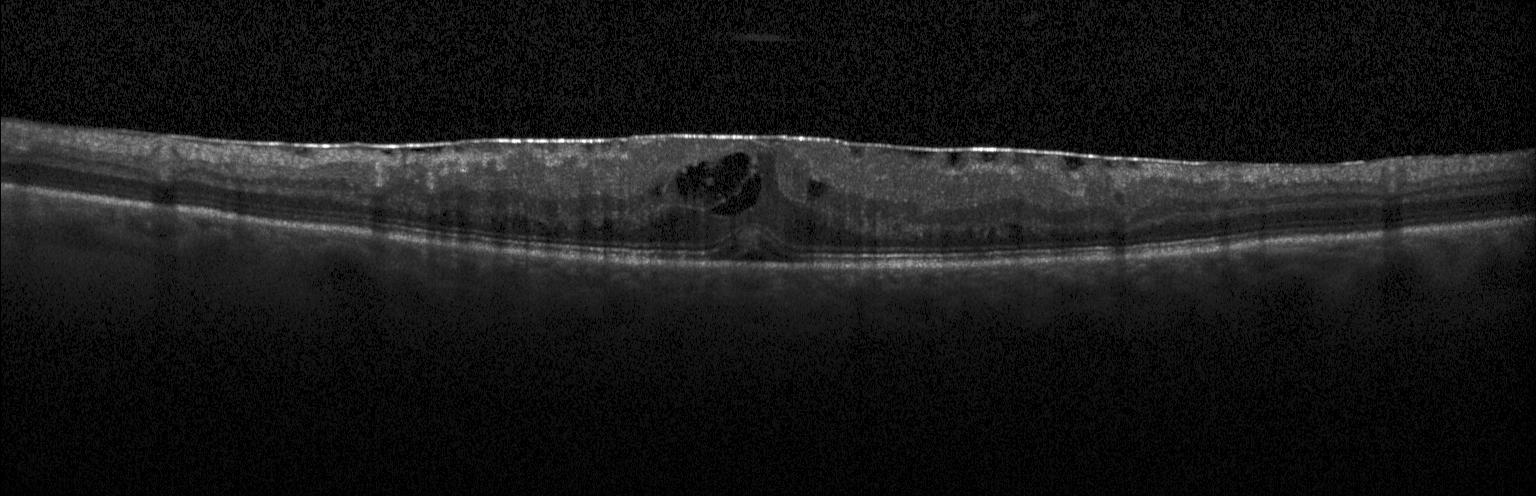
OCT scan showing DME.